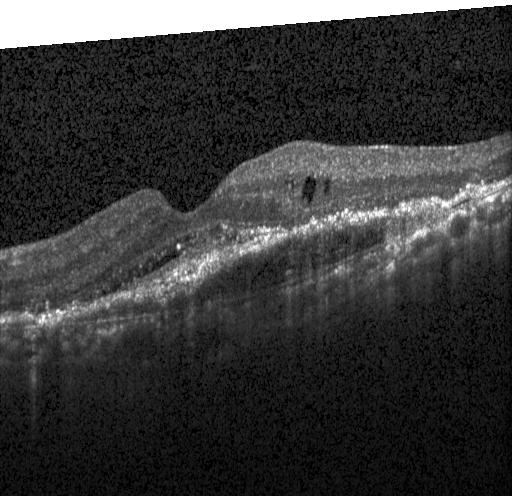

OCT scan showing choroidal neovascularization (CNV).